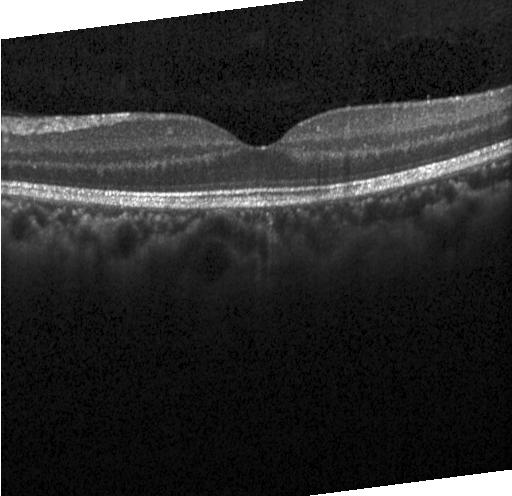

No choroidal neovascularization, diabetic macular edema, or drusen.